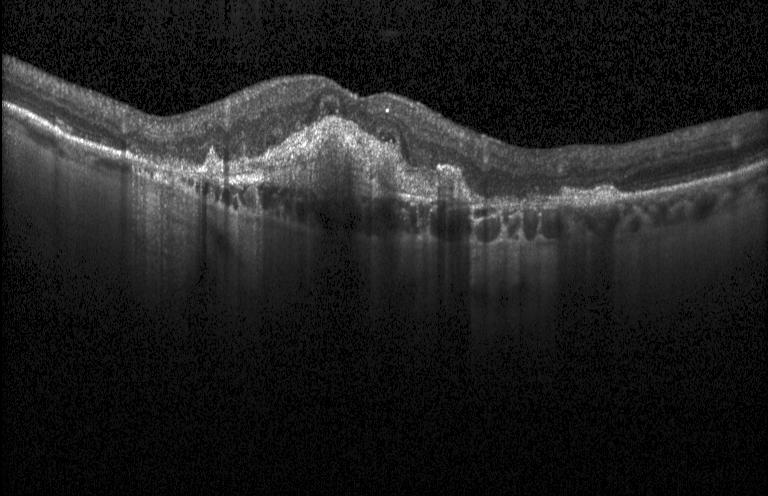

A choroidal neovascular membrane.